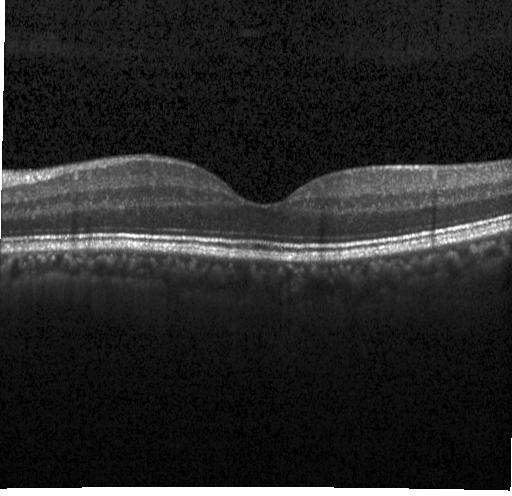 OCT B-scan — Diagnosis: no CNV, no DME, and no drusen.